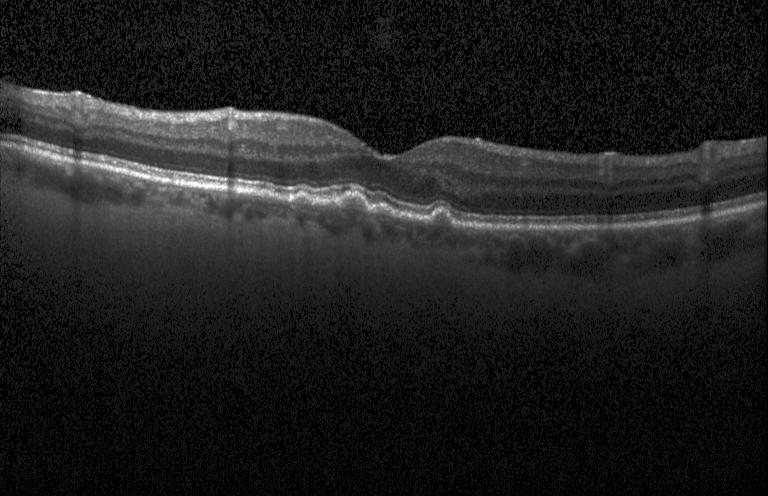
OCT B-scan showing multiple drusen.